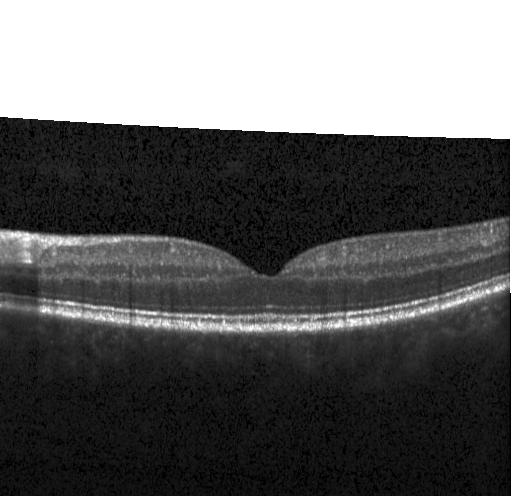 Spectral-domain optical coherence tomography. Instrument: Heidelberg Spectralis. Horizontal scan through the fovea. OCT B-scan — Finding: no evidence of choroidal neovascularization, diabetic macular edema, or drusen.